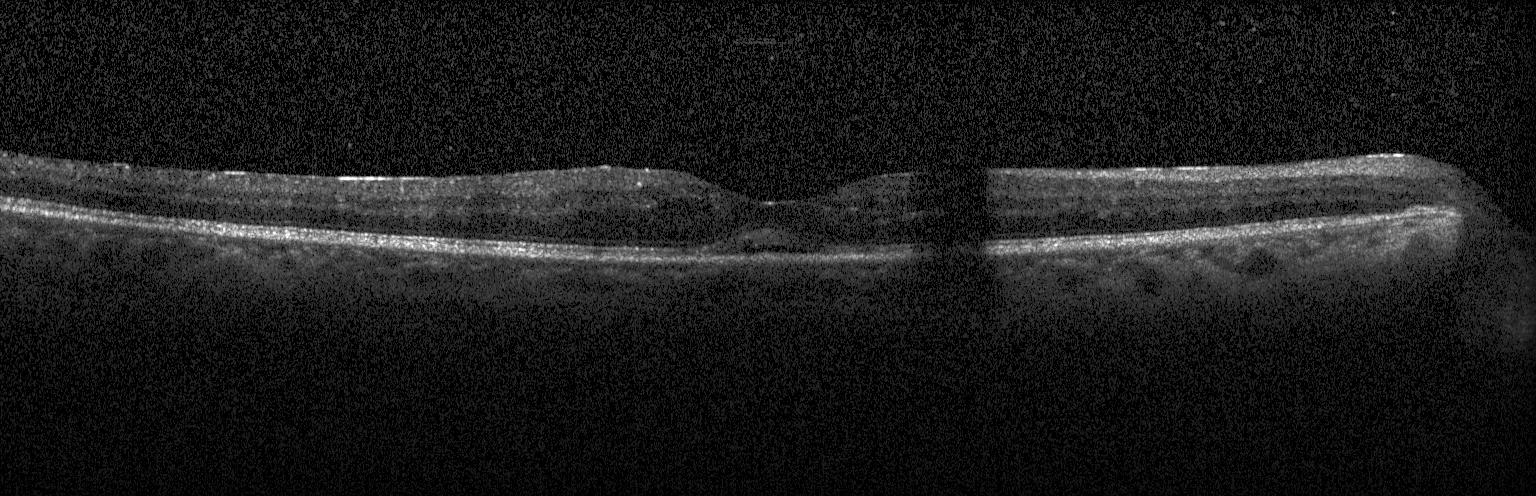
No evidence of choroidal neovascularization, diabetic macular edema, or drusen.